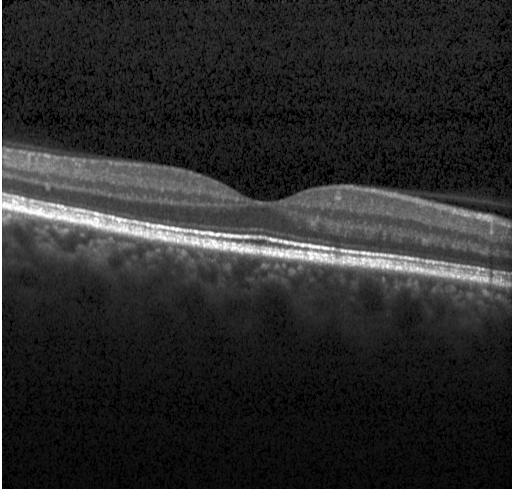

Impression: no choroidal neovascularization, no diabetic macular edema, and no drusen.